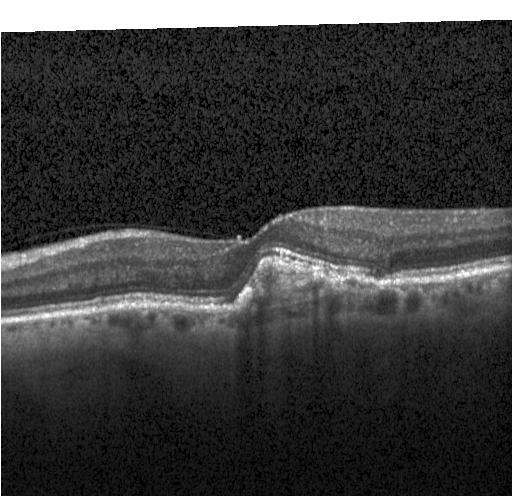

OCT line scan.
The scan shows choroidal neovascularization (CNV).